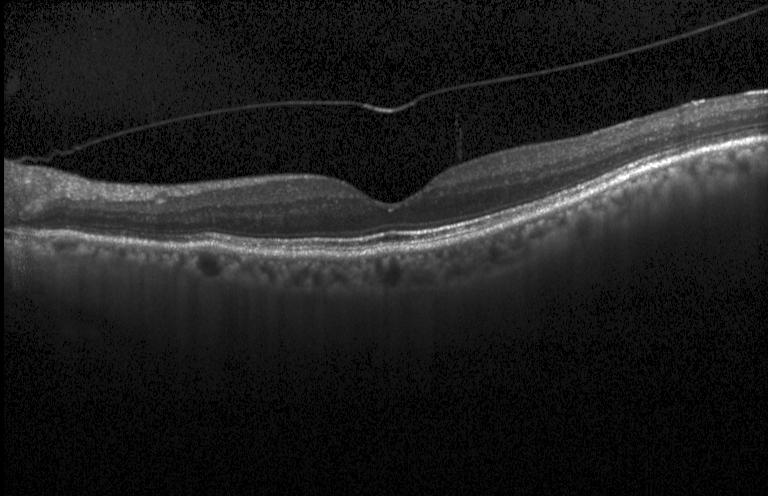
Diagnosis: neither choroidal neovascularization, diabetic macular edema, nor drusen.